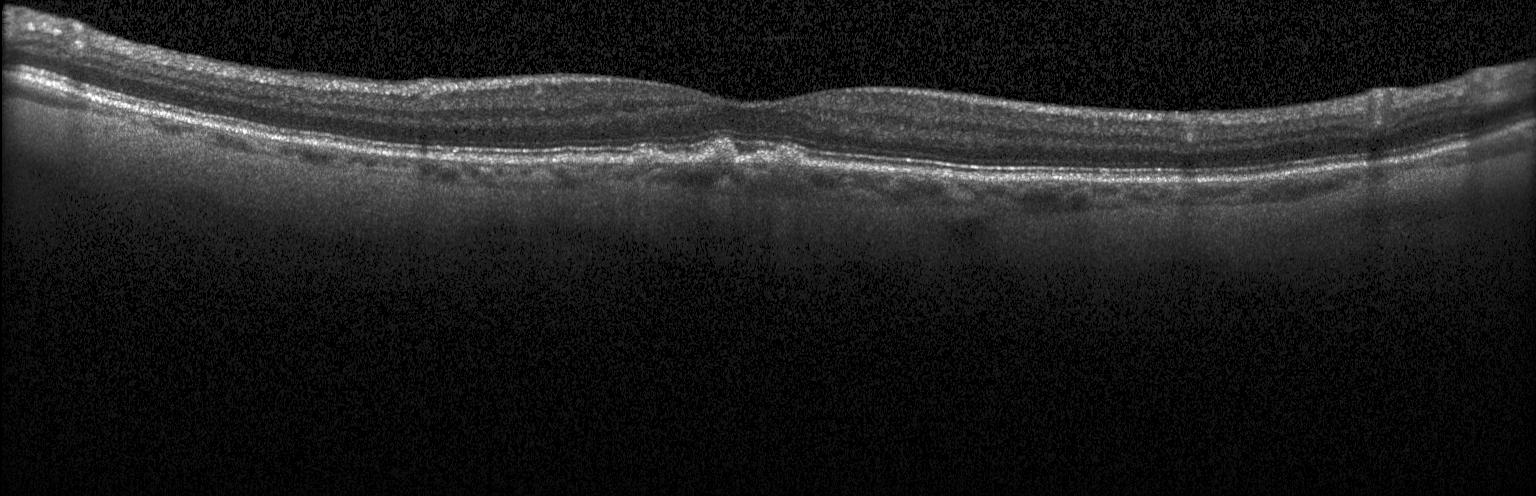
Centered on the fovea, optical coherence tomography B-scan
Multiple drusen.